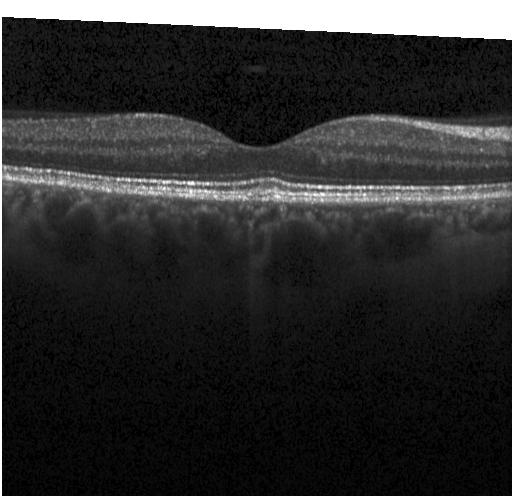

Centered on the fovea · acquired on a Heidelberg Spectralis · optical coherence tomography B-scan
Finding: no choroidal neovascularization, no diabetic macular edema, and no drusen.